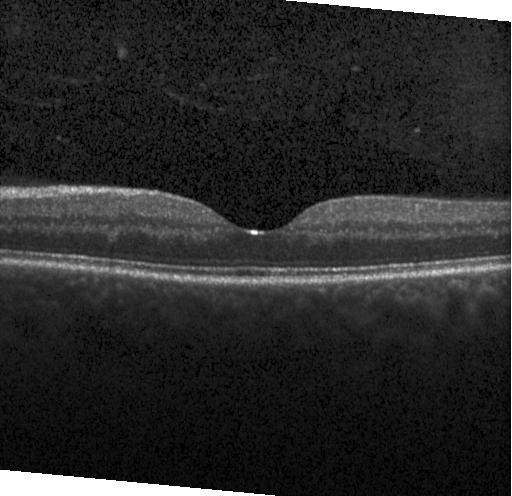 OCT line scan. Through the macula. Spectral-domain OCT. Instrument: Heidelberg Spectralis.
The scan shows no evidence of choroidal neovascularization, diabetic macular edema, or drusen.